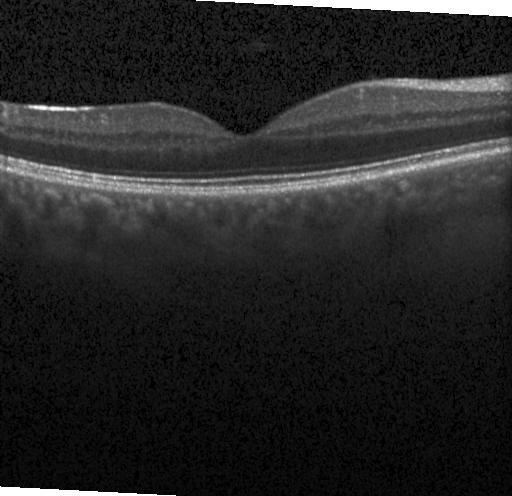 Fovea-centered. Retinal OCT cross-section. Heidelberg Spectralis. SD-OCT. Diagnosis: neither choroidal neovascularization, diabetic macular edema, nor drusen.